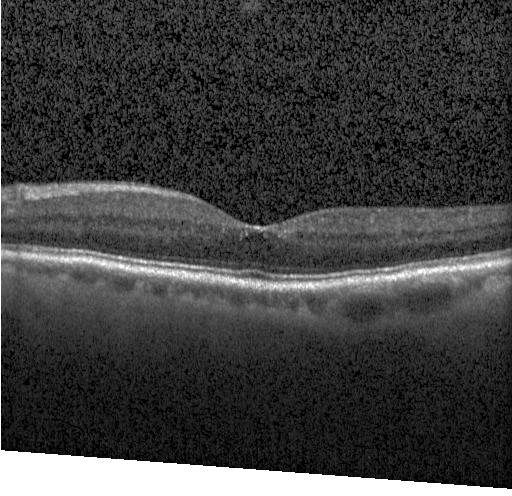

Fovea-centered · optical coherence tomography scan · spectral-domain optical coherence tomography · Heidelberg Spectralis — Dx: no evidence of CNV, DME, or drusen.